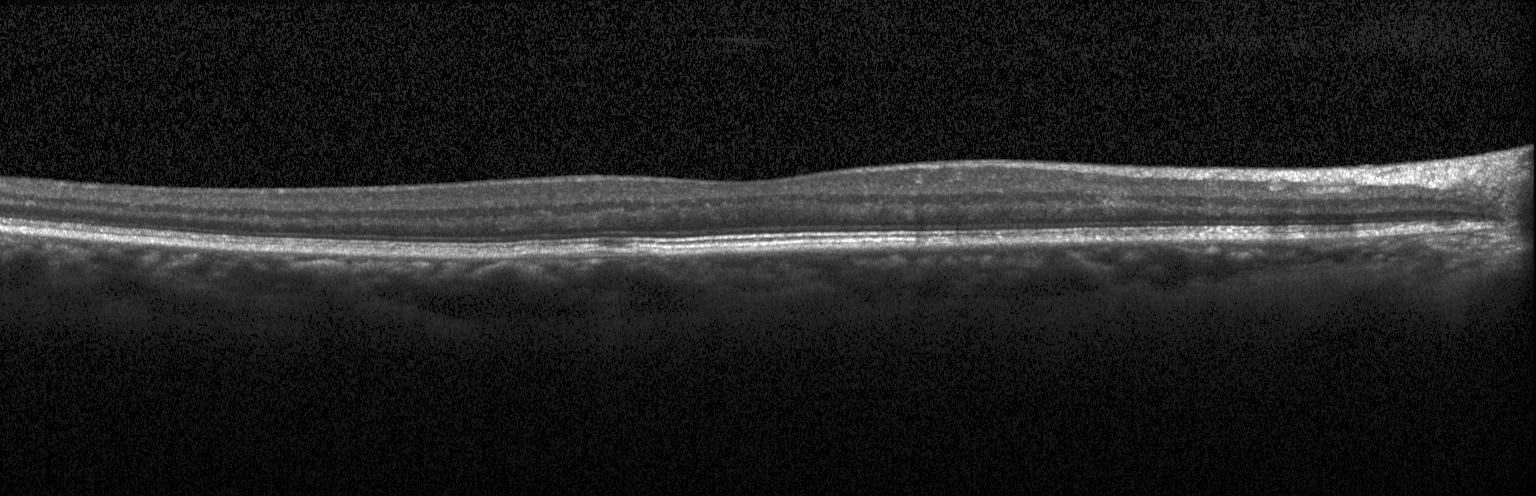
Spectral-domain OCT. OCT B-scan
Finding: no evidence of CNV, DME, or drusen.